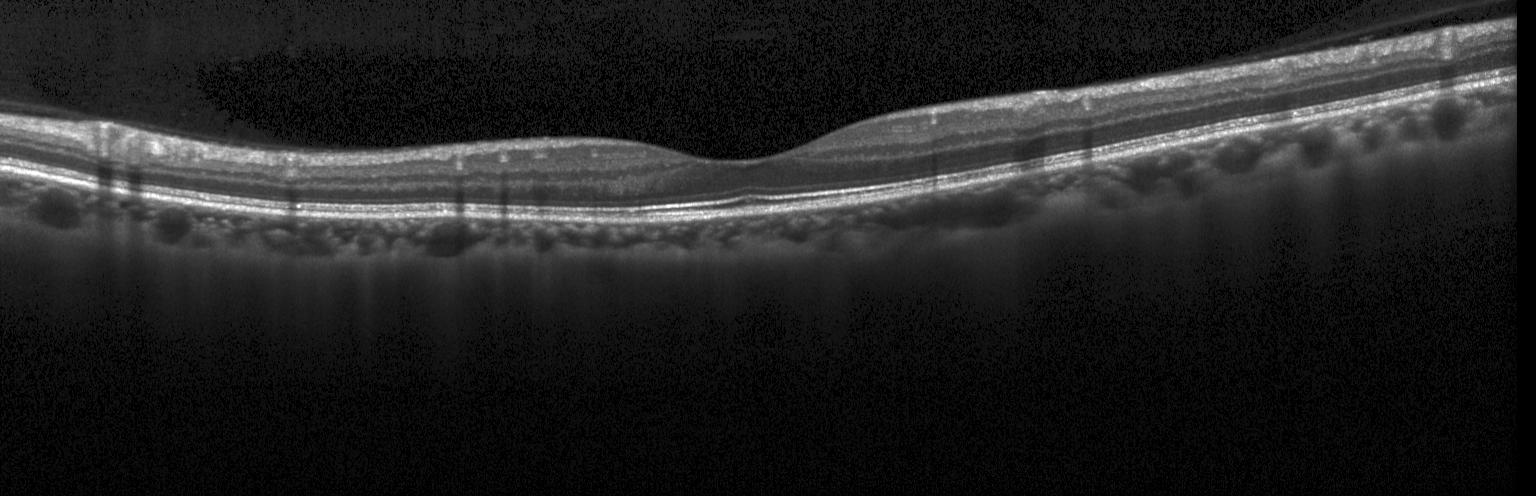 Optical coherence tomography scan; Heidelberg Spectralis OCT system
Dx: no CNV, DME, or drusen.